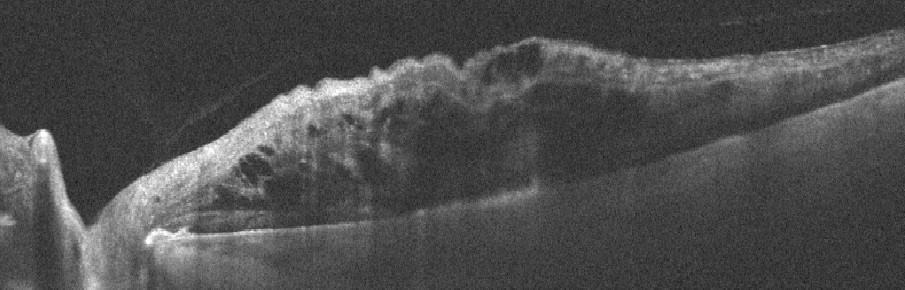 Optical coherence tomography scan
Macular OCT: retinal vein occlusion.